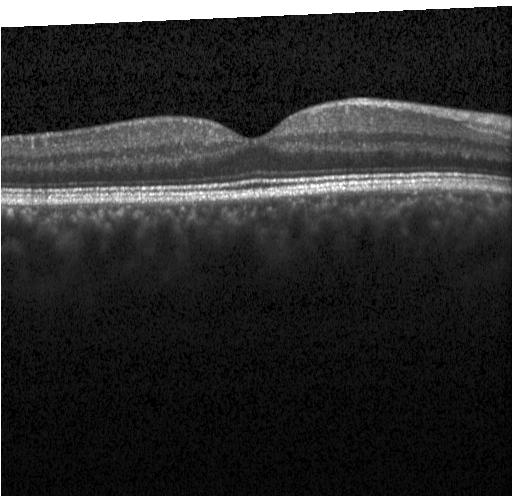 Spectral-domain OCT B-scan: no choroidal neovascularization, no diabetic macular edema, and no drusen.